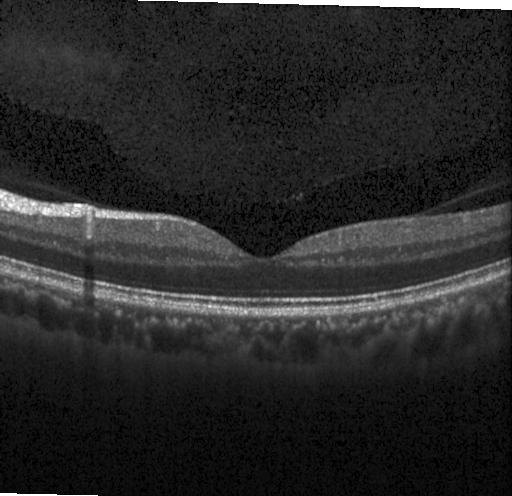

Dx: no choroidal neovascularization, diabetic macular edema, or drusen.